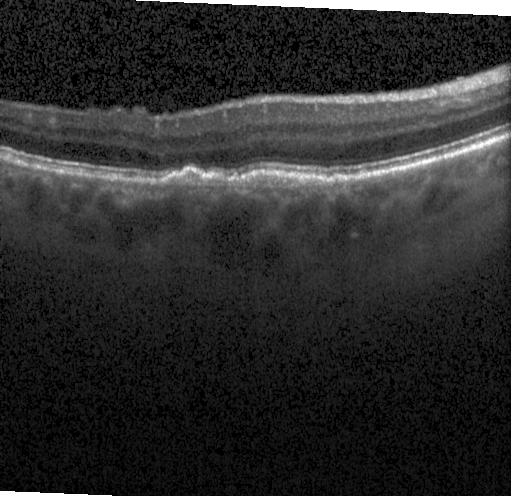

Horizontal scan through the fovea · optical coherence tomography B-scan · Heidelberg Spectralis · SD-OCT. Impression: choroidal neovascularization (CNV).